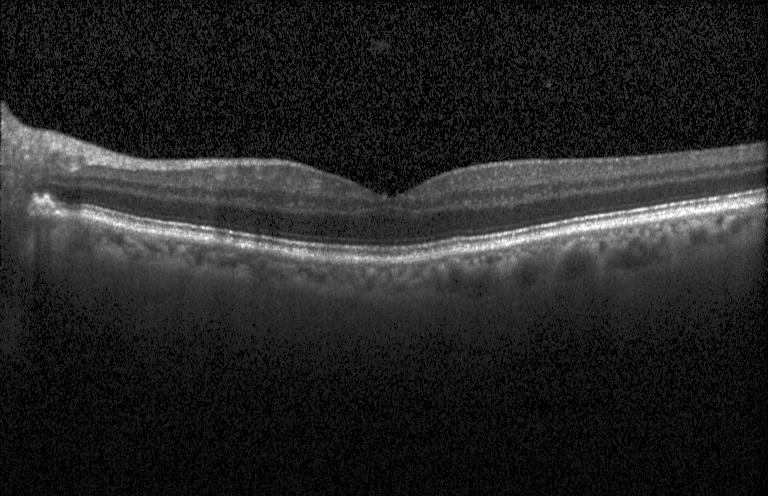
Spectral-domain OCT, fovea-centered, acquired on a Heidelberg Spectralis, retinal OCT B-scan. Assessment: neither choroidal neovascularization, diabetic macular edema, nor drusen.